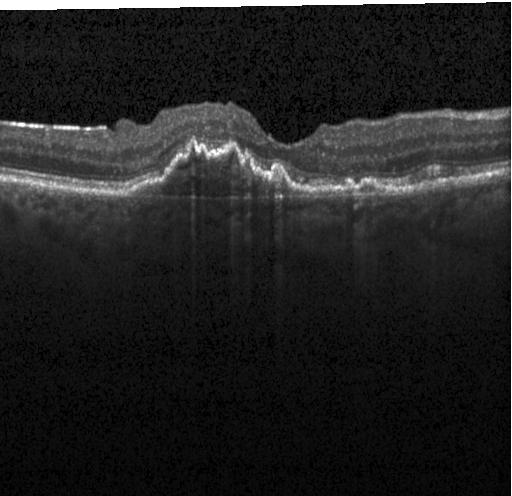 Spectral-domain OCT; optical coherence tomography scan; centered on the fovea; Heidelberg Spectralis.
Impression: a choroidal neovascular membrane.